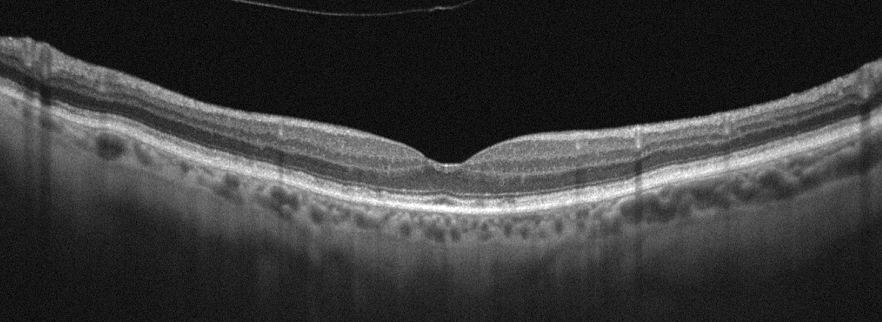
Finding: age-related macular degeneration (AMD).